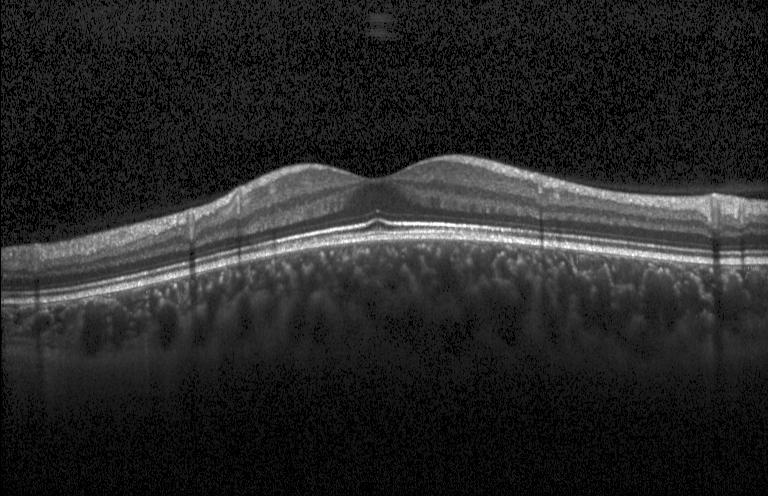
Instrument: Heidelberg Spectralis · centered on the fovea · retinal OCT B-scan.
Finding: no CNV, no DME, and no drusen.